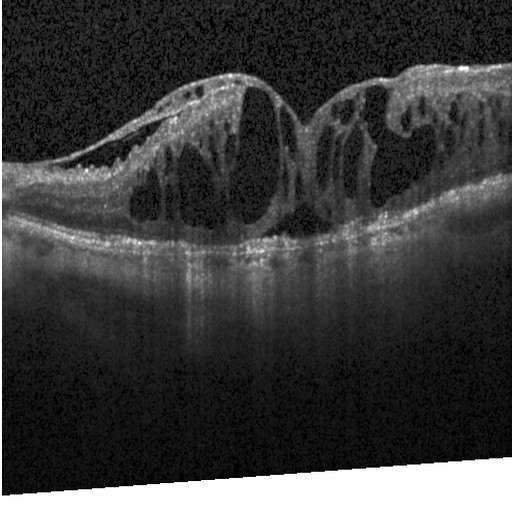
Retinal OCT cross-section
Diabetic macular edema (DME).